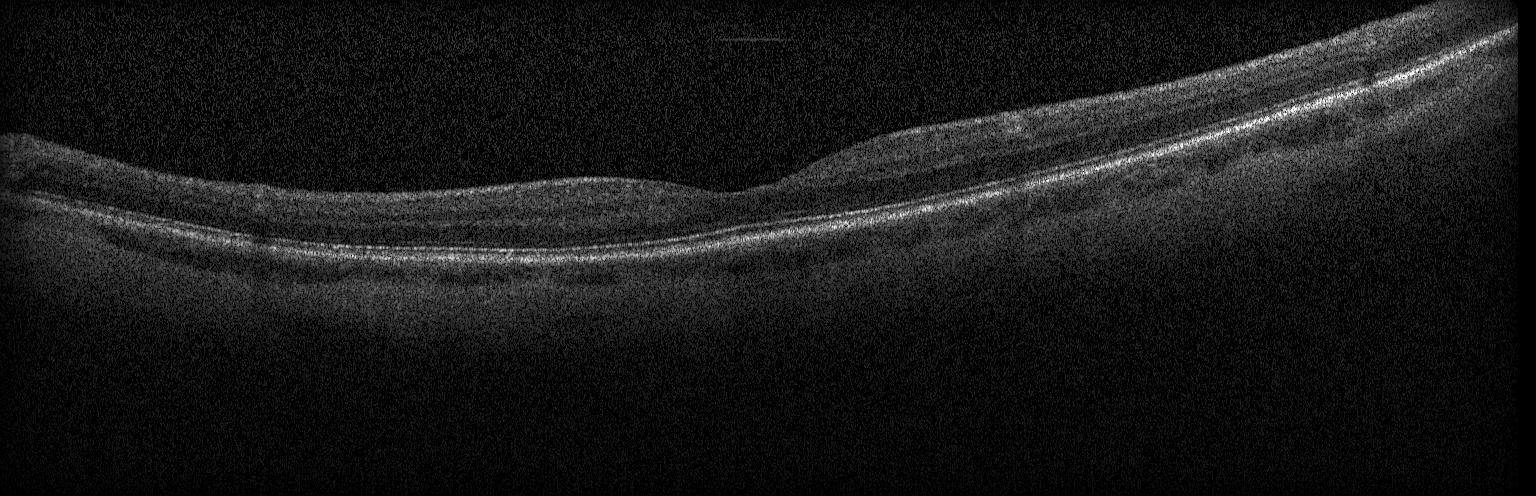 OCT finding: no evidence of choroidal neovascularization, diabetic macular edema, or drusen.